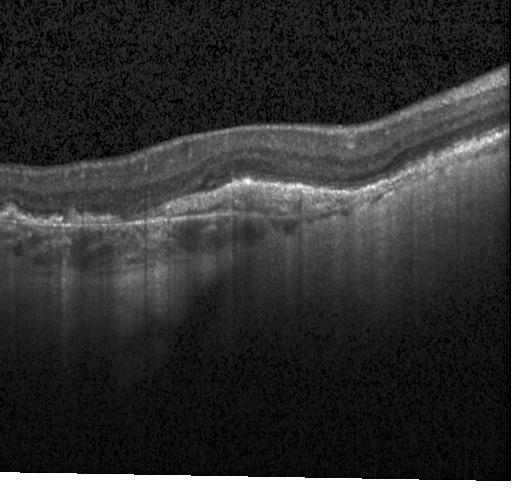
Finding: choroidal neovascularization.